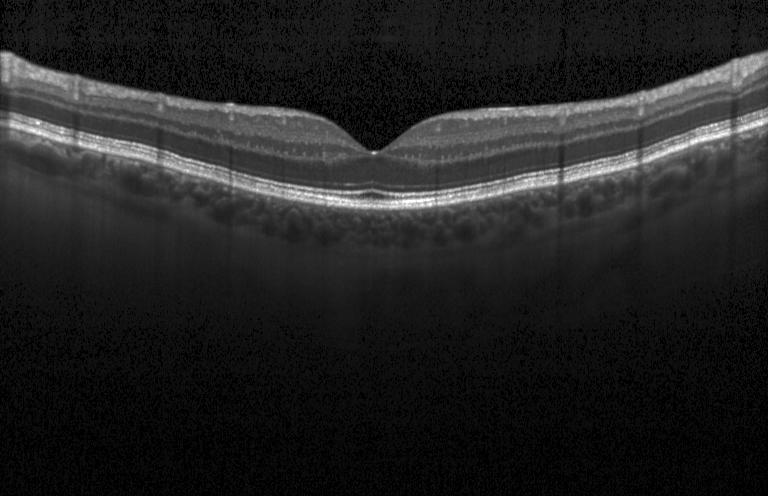 Through the macula. Acquired on a Heidelberg Spectralis. OCT line scan. Spectral-domain optical coherence tomography — OCT finding: no choroidal neovascularization, diabetic macular edema, or drusen.